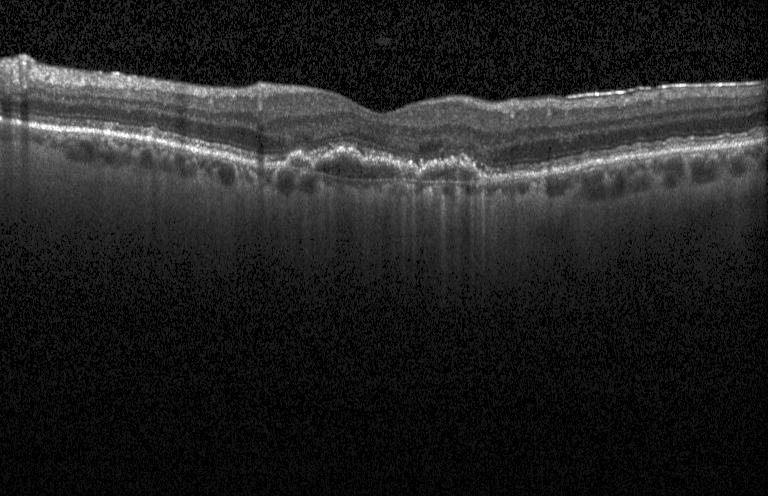

Horizontal scan through the fovea; instrument: Heidelberg Spectralis; retinal OCT cross-section.
Diagnosis: CNV.